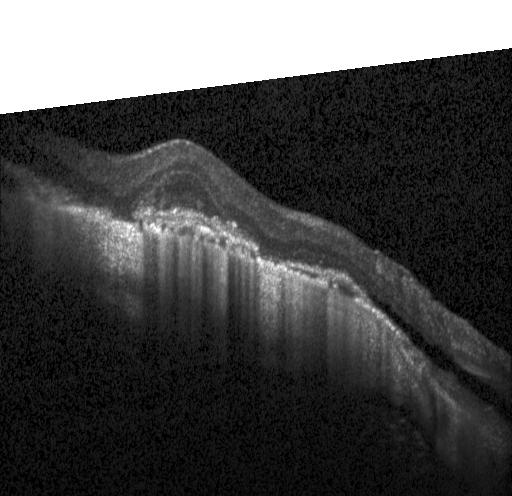
Spectral-domain optical coherence tomography. Through the macula. Optical coherence tomography scan. Instrument: Heidelberg Spectralis
Impression: choroidal neovascularization (CNV).